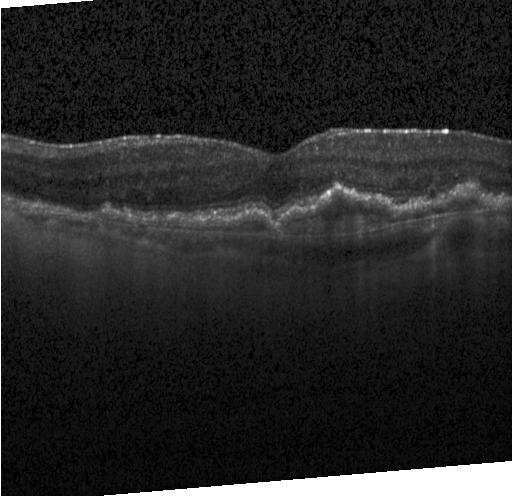

Spectral-domain OCT B-scan: choroidal neovascularization.